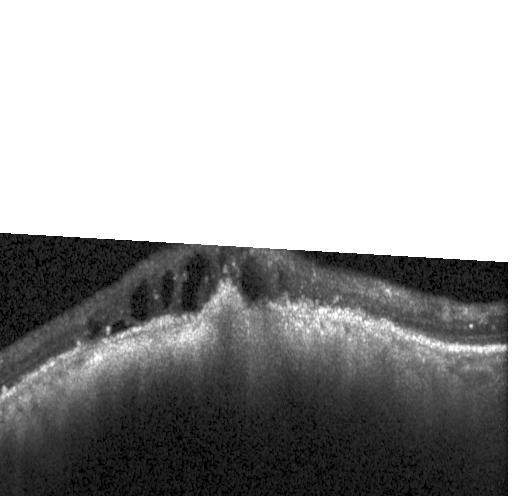 Spectral-domain OCT B-scan: choroidal neovascularization.